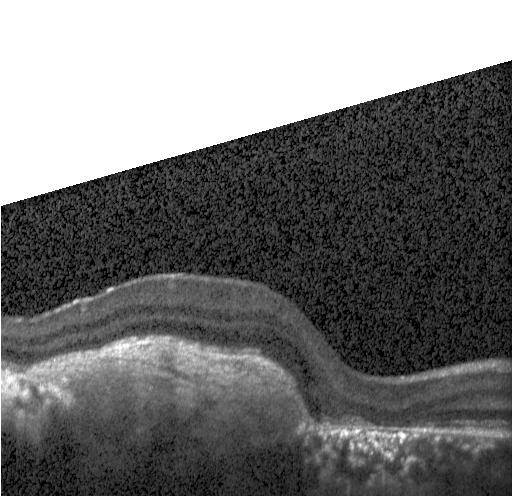 Optical coherence tomography scan. Spectral-domain OCT.
Assessment: a choroidal neovascular membrane.